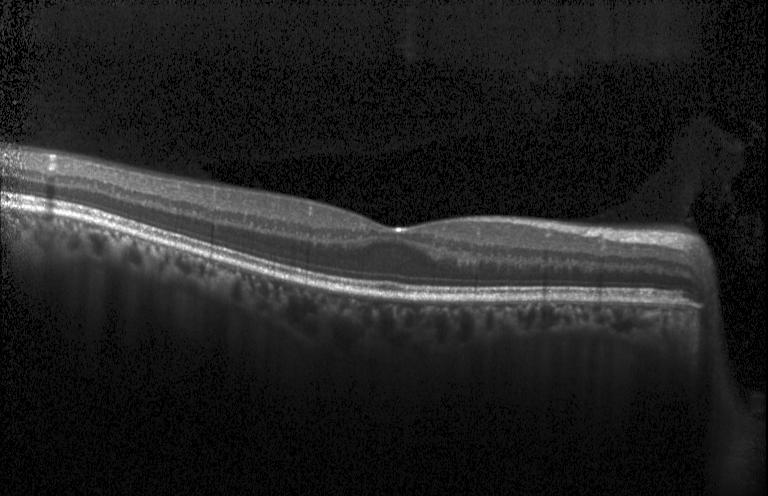

OCT line scan · macular scan · SD-OCT · acquired on a Heidelberg Spectralis.
Dx: neither choroidal neovascularization, diabetic macular edema, nor drusen.